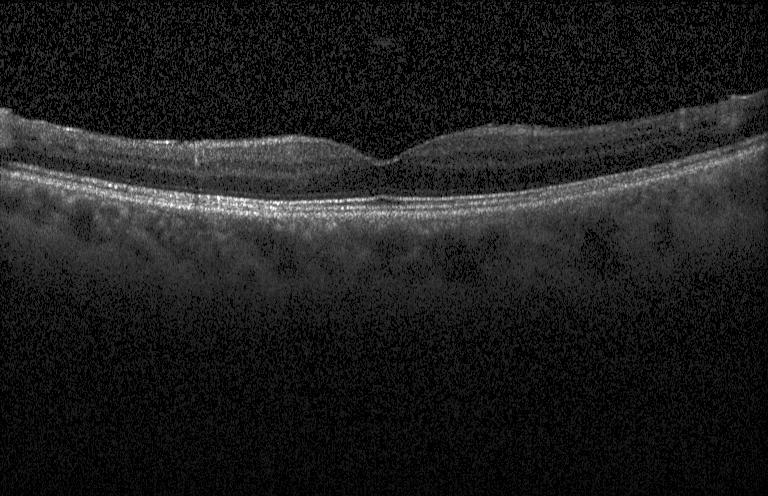

OCT line scan; horizontal scan through the fovea; Heidelberg Spectralis OCT system. Diagnosis: no evidence of choroidal neovascularization, diabetic macular edema, or drusen.